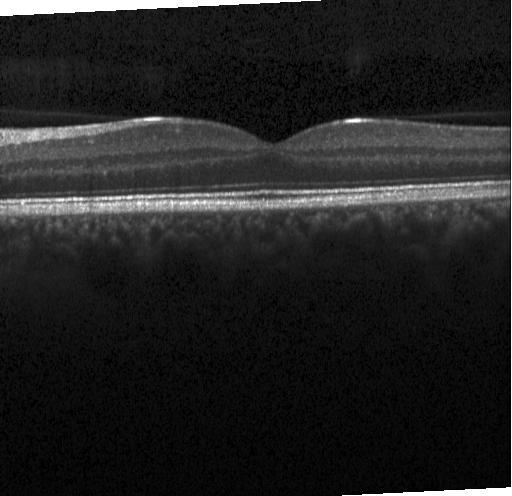
OCT B-scan showing no evidence of choroidal neovascularization, diabetic macular edema, or drusen.